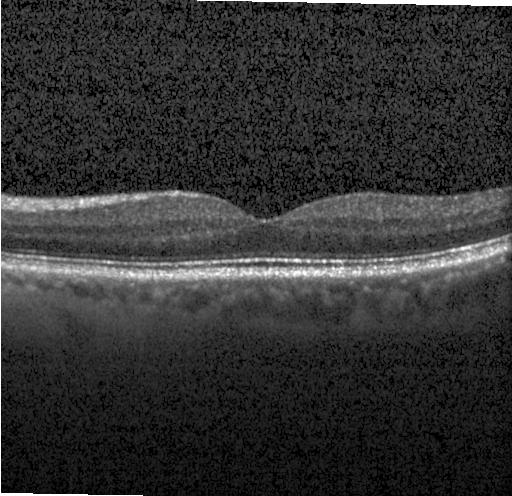
Spectral-domain optical coherence tomography, OCT B-scan. Diagnosis: neither choroidal neovascularization, diabetic macular edema, nor drusen.